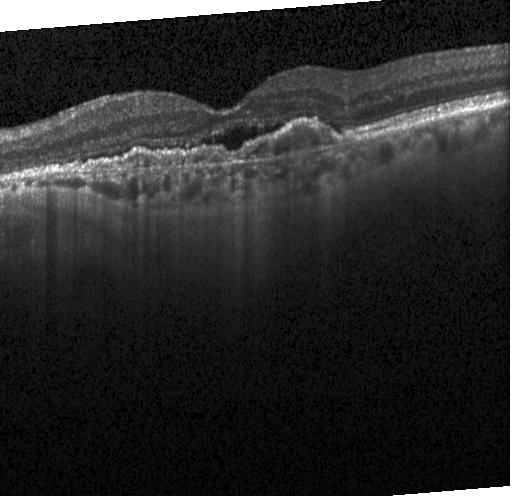
Through the macula. OCT B-scan. Instrument: Heidelberg Spectralis — Macular OCT: choroidal neovascularization.